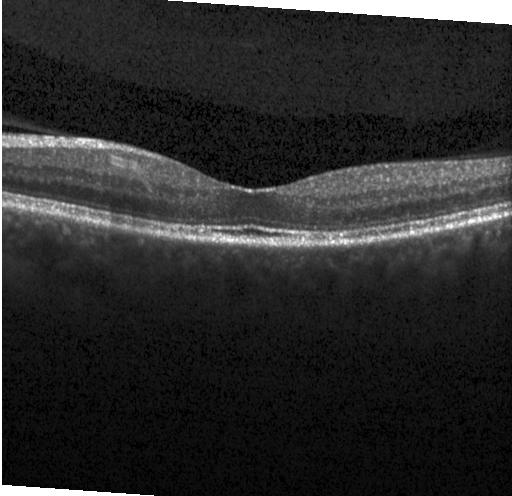 Horizontal scan through the fovea · SD-OCT · OCT B-scan · Heidelberg Spectralis. This B-scan demonstrates no choroidal neovascularization, no diabetic macular edema, and no drusen.